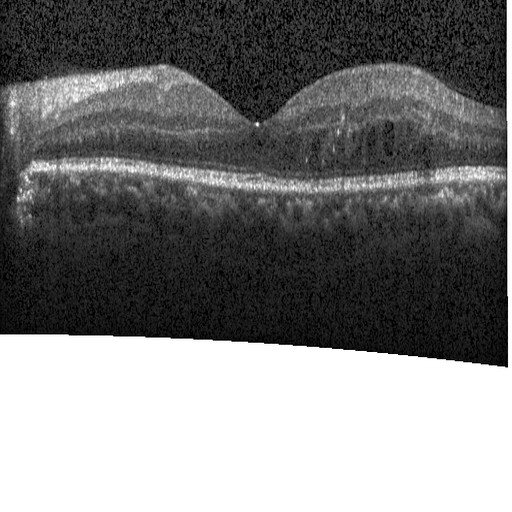

Retinal OCT B-scan — OCT finding: diabetic macular edema (DME).